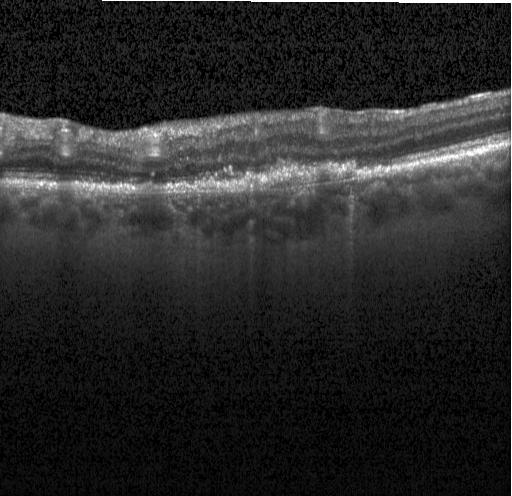

OCT B-scan; spectral-domain OCT; acquired on a Heidelberg Spectralis.
Impression: a choroidal neovascular membrane.